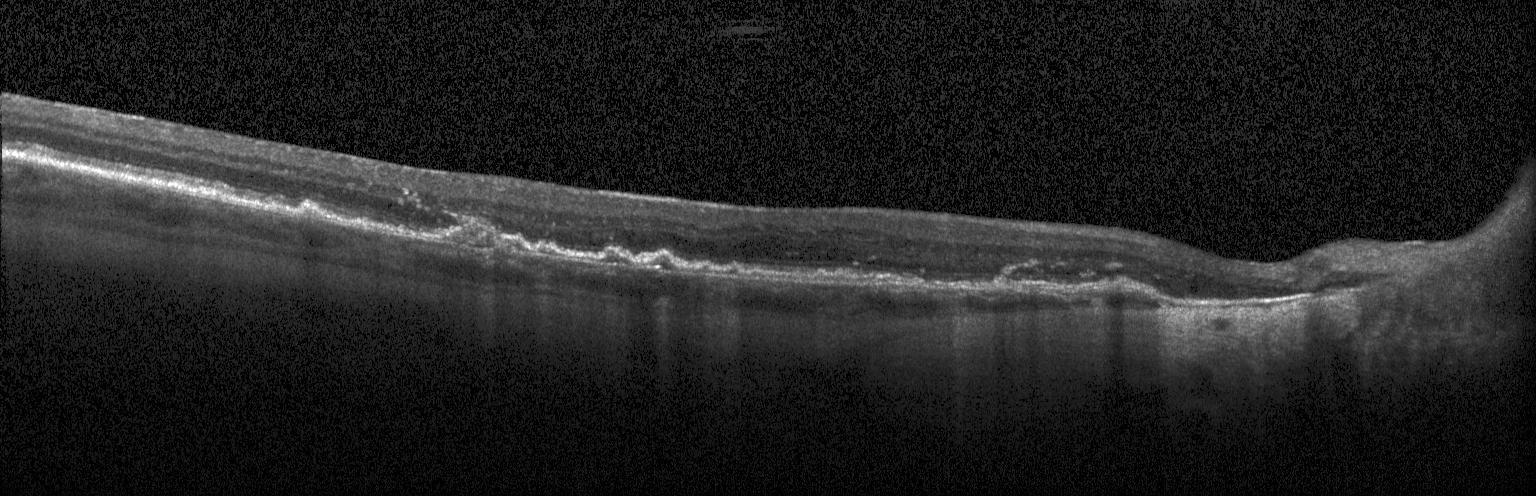
OCT line scan
This B-scan demonstrates a choroidal neovascular membrane.